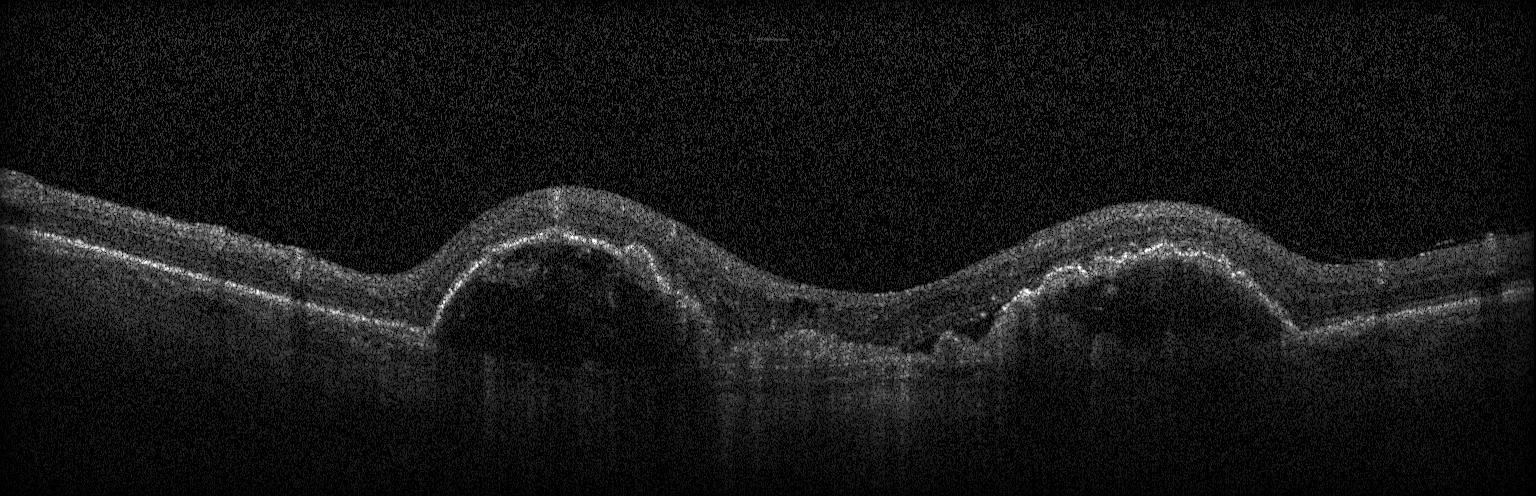 OCT finding: a choroidal neovascular membrane.